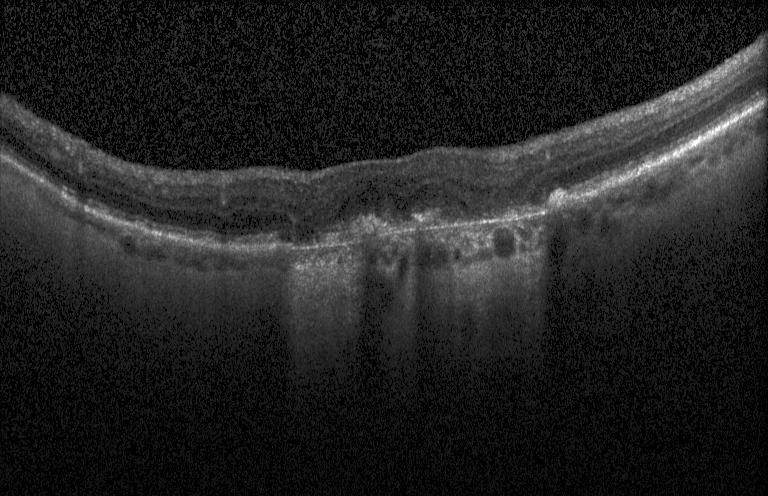
OCT scan showing a choroidal neovascular membrane.